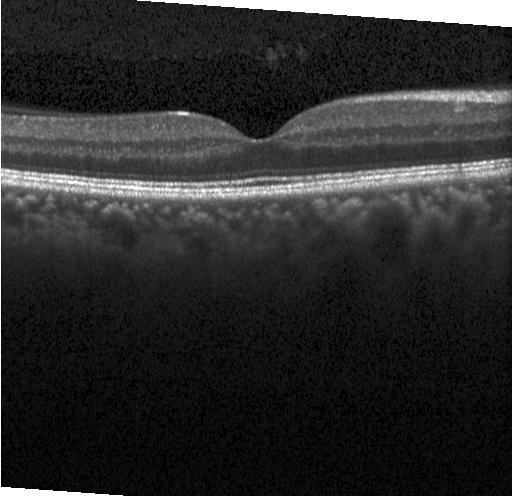 Retinal OCT B-scan; macular scan
Diagnosis: neither choroidal neovascularization, diabetic macular edema, nor drusen.